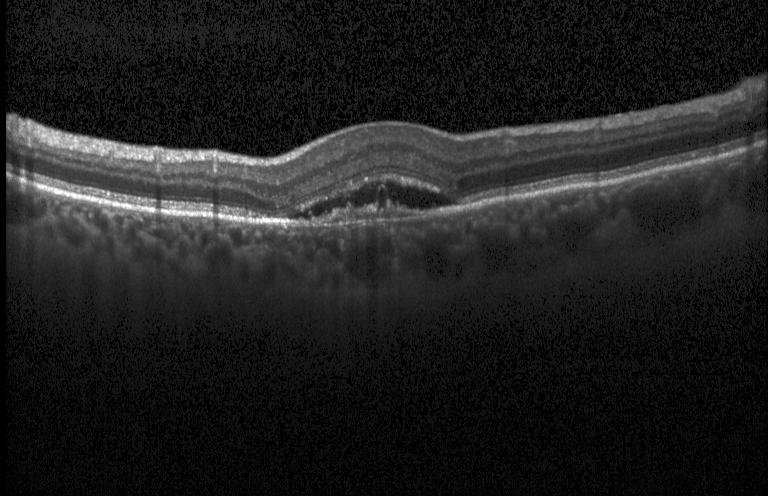

Through the macula; optical coherence tomography scan; acquired on a Heidelberg Spectralis — Impression: a choroidal neovascular membrane.